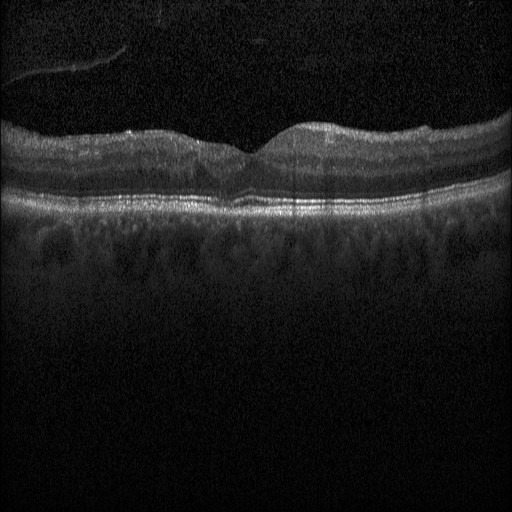 Finding: DME.